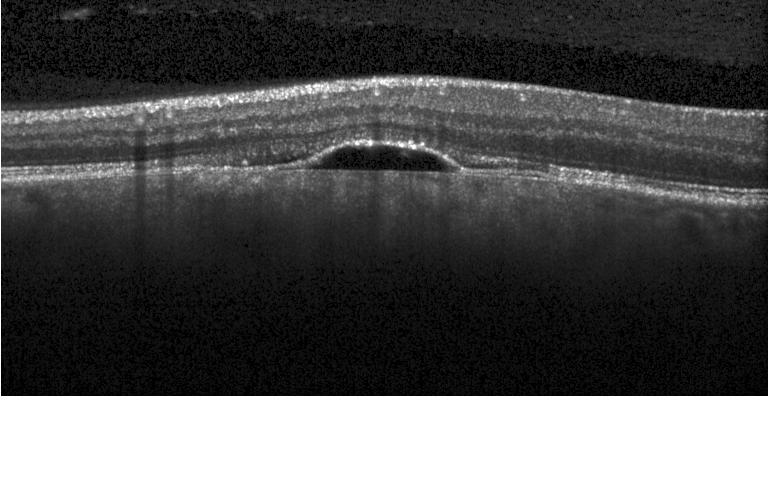 Impression: choroidal neovascularization.